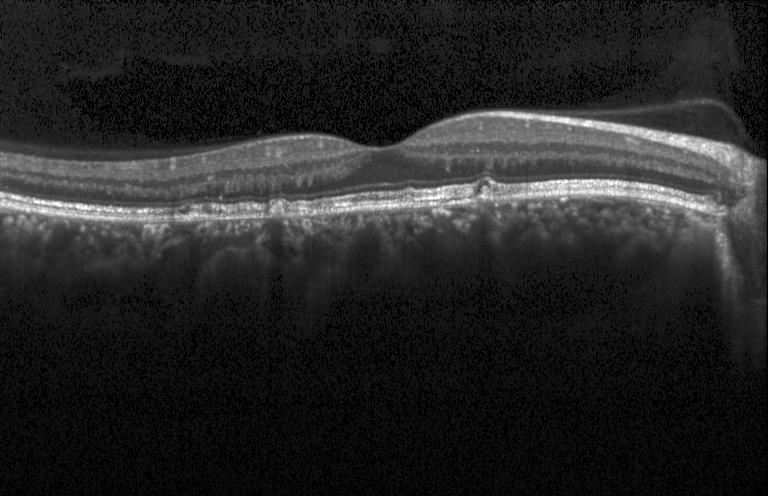

Diagnosis: sub-RPE drusenoid deposits.